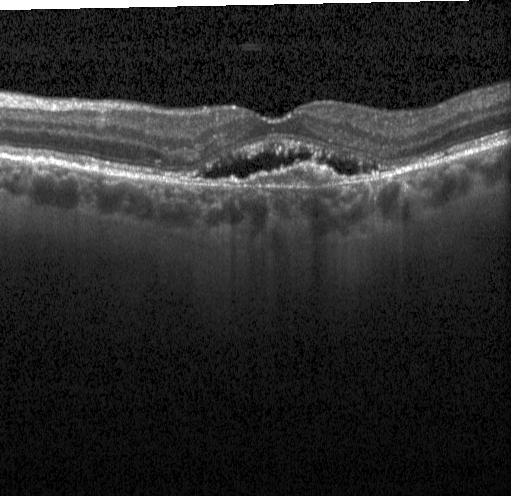

Impression: a choroidal neovascular membrane.